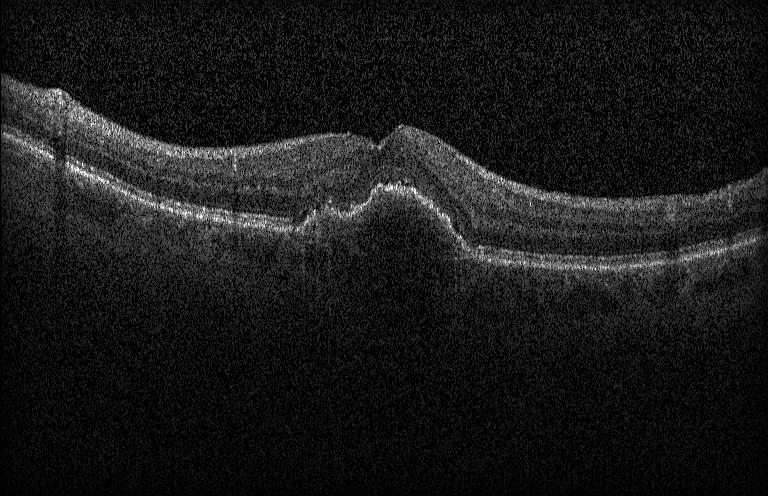 Dx: a choroidal neovascular membrane.